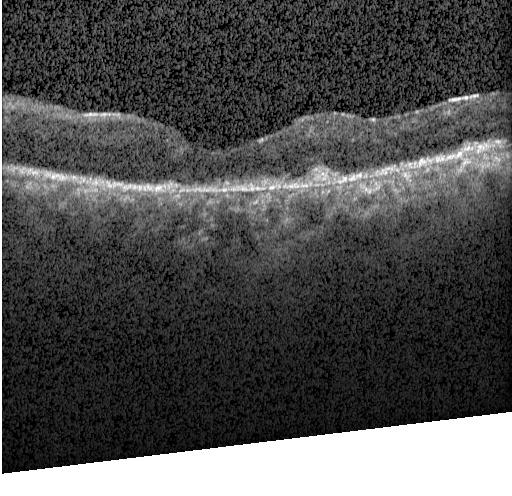
This B-scan demonstrates choroidal neovascularization.